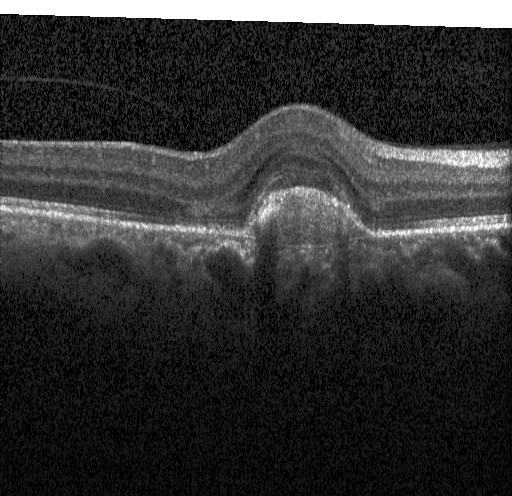 Diagnosis: CNV.